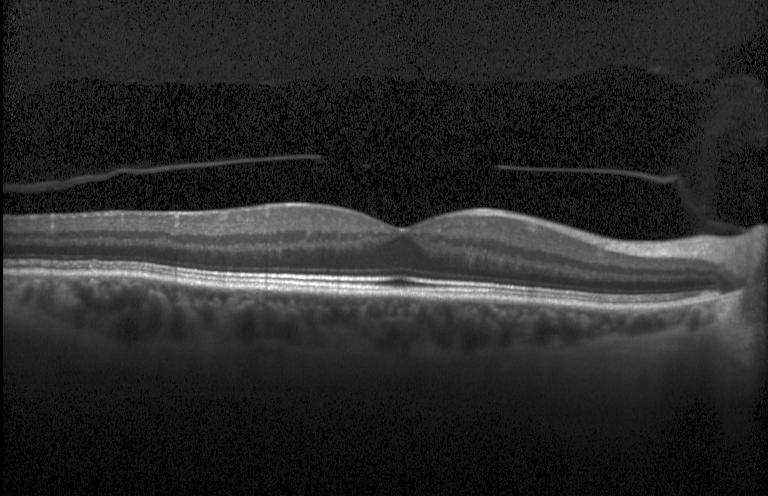
Optical coherence tomography B-scan. Horizontal scan through the fovea. Heidelberg Spectralis — The scan shows no choroidal neovascularization, no diabetic macular edema, and no drusen.